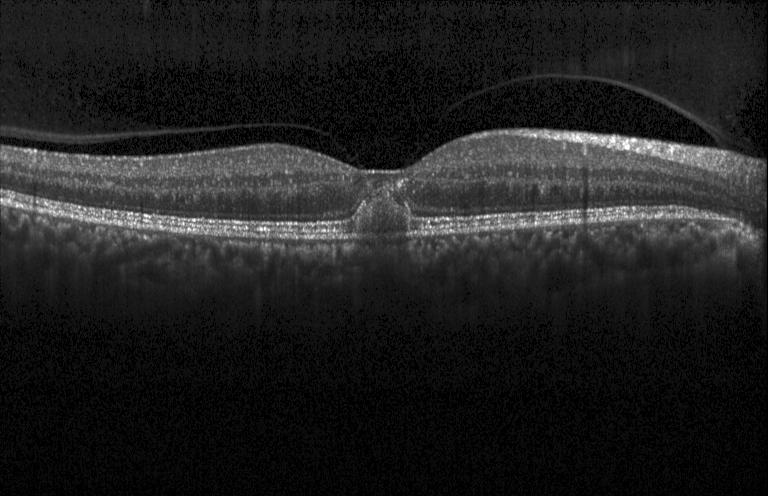
Instrument: Heidelberg Spectralis; through the macula; optical coherence tomography B-scan; spectral-domain OCT.
Finding: CNV.